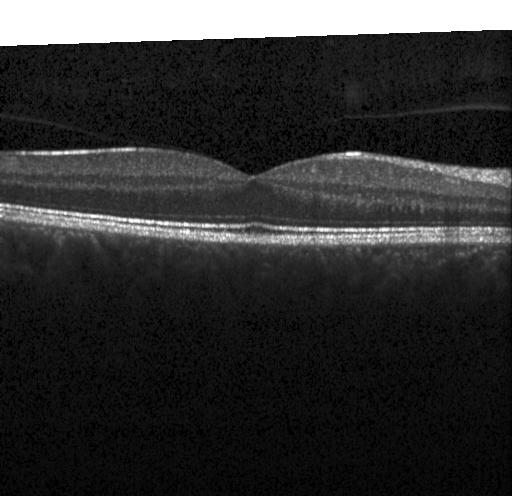
OCT line scan — Dx: no choroidal neovascularization, diabetic macular edema, or drusen.